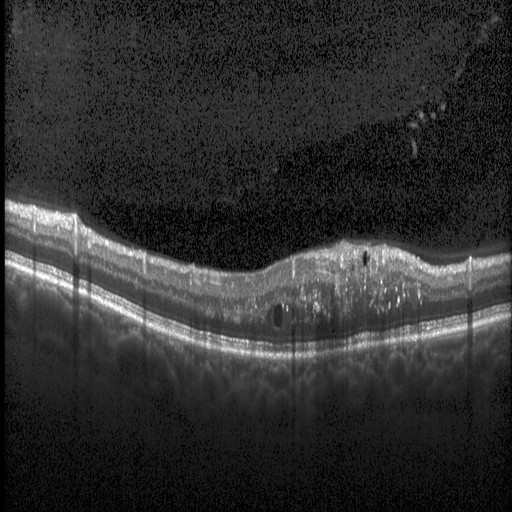

Spectral-domain optical coherence tomography · retinal OCT cross-section. OCT finding: diabetic macular edema (DME).